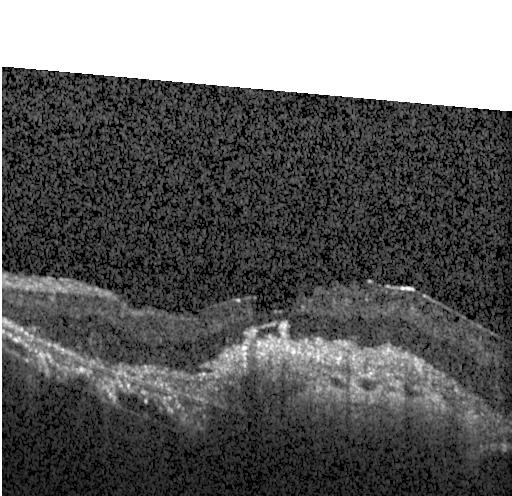
Spectral-domain OCT B-scan: a choroidal neovascular membrane.